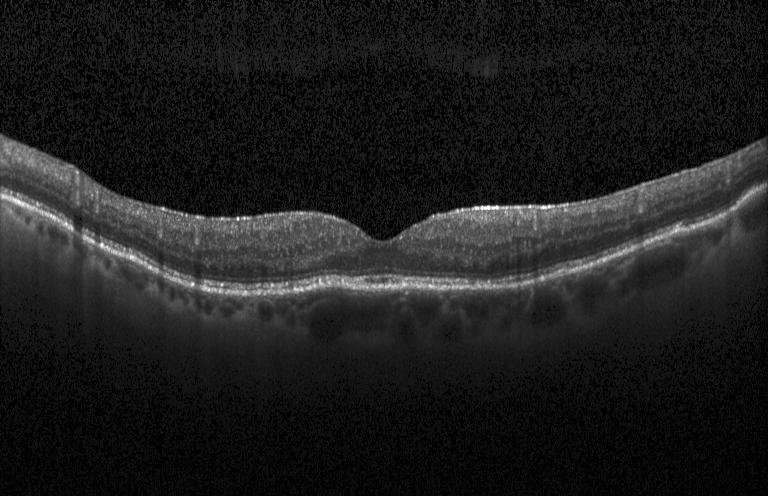 This B-scan demonstrates no evidence of choroidal neovascularization, diabetic macular edema, or drusen.